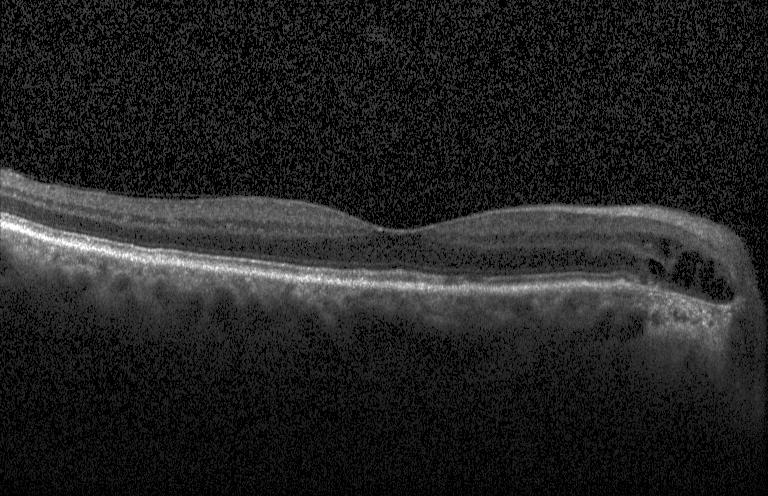
SD-OCT, OCT line scan, horizontal scan through the fovea.
Diabetic macular edema.